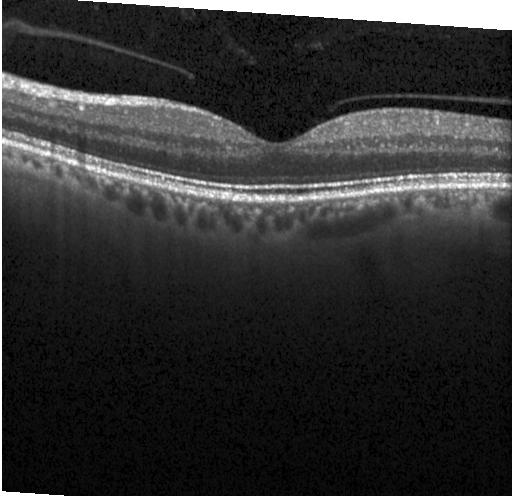

Retinal OCT B-scan. Diagnosis: no evidence of CNV, DME, or drusen.